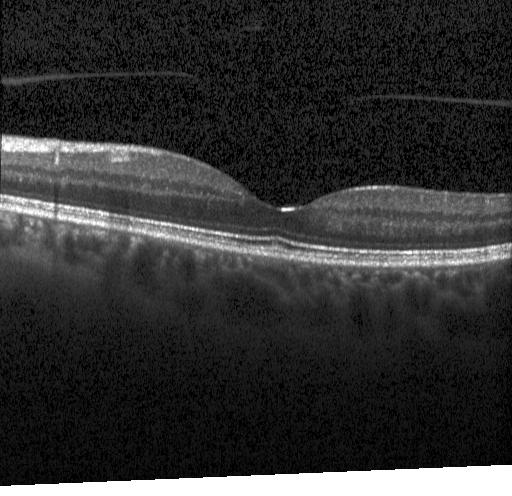
Macular scan; retinal OCT B-scan
Diagnosis: no evidence of choroidal neovascularization, diabetic macular edema, or drusen.